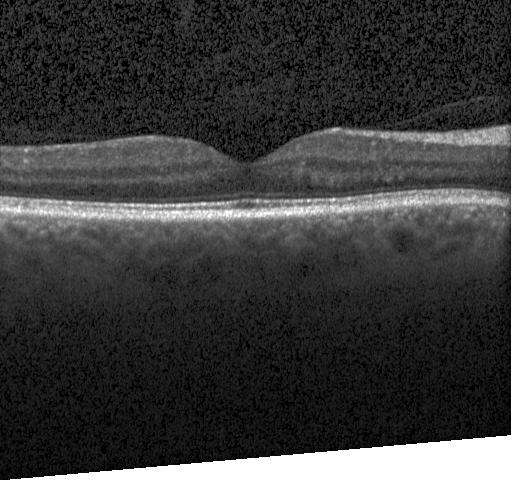
OCT B-scan. Finding: no evidence of CNV, DME, or drusen.